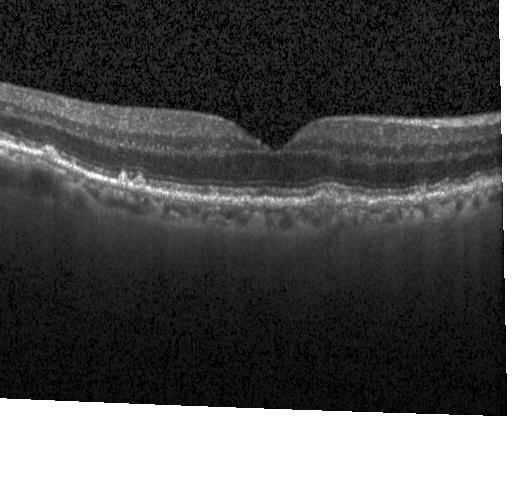

Heidelberg Spectralis OCT system, retinal OCT cross-section.
This B-scan demonstrates drusen.